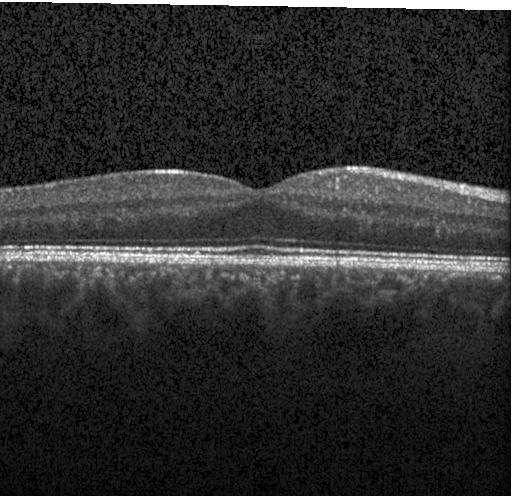 OCT B-scan showing no CNV, DME, or drusen.